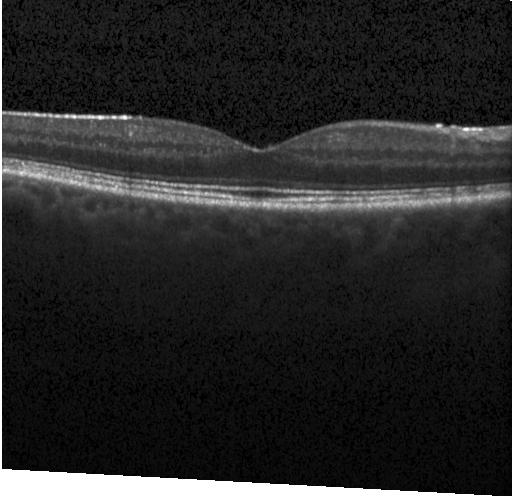

Finding: no choroidal neovascularization, no diabetic macular edema, and no drusen.